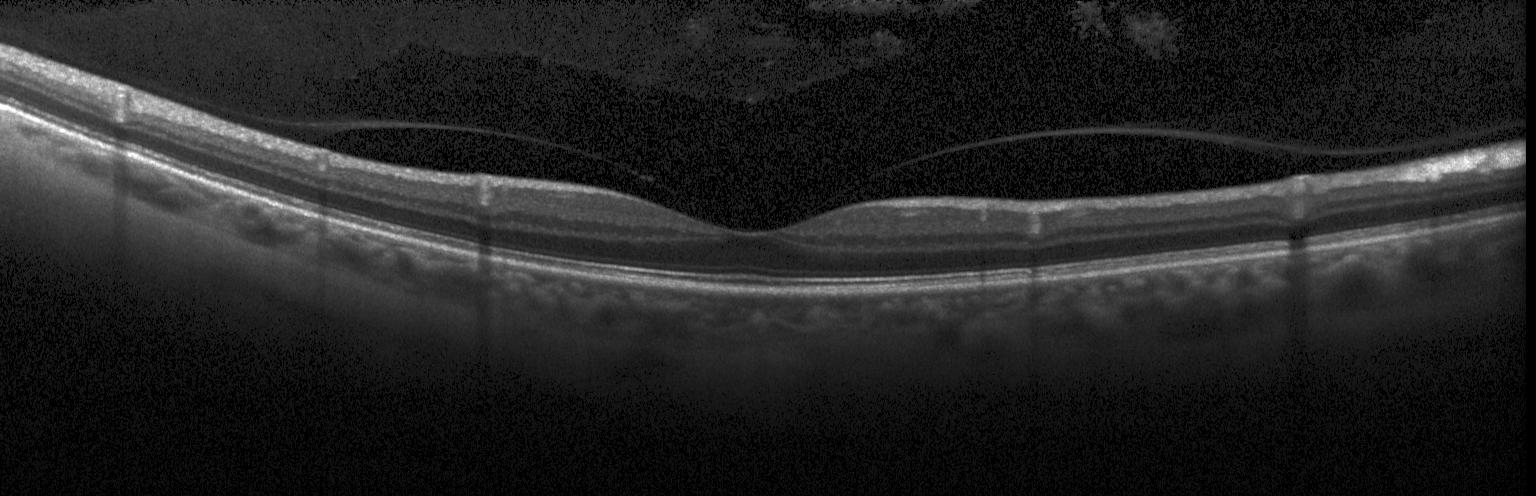

Through the macula · Heidelberg Spectralis · OCT B-scan
Dx: no evidence of choroidal neovascularization, diabetic macular edema, or drusen.